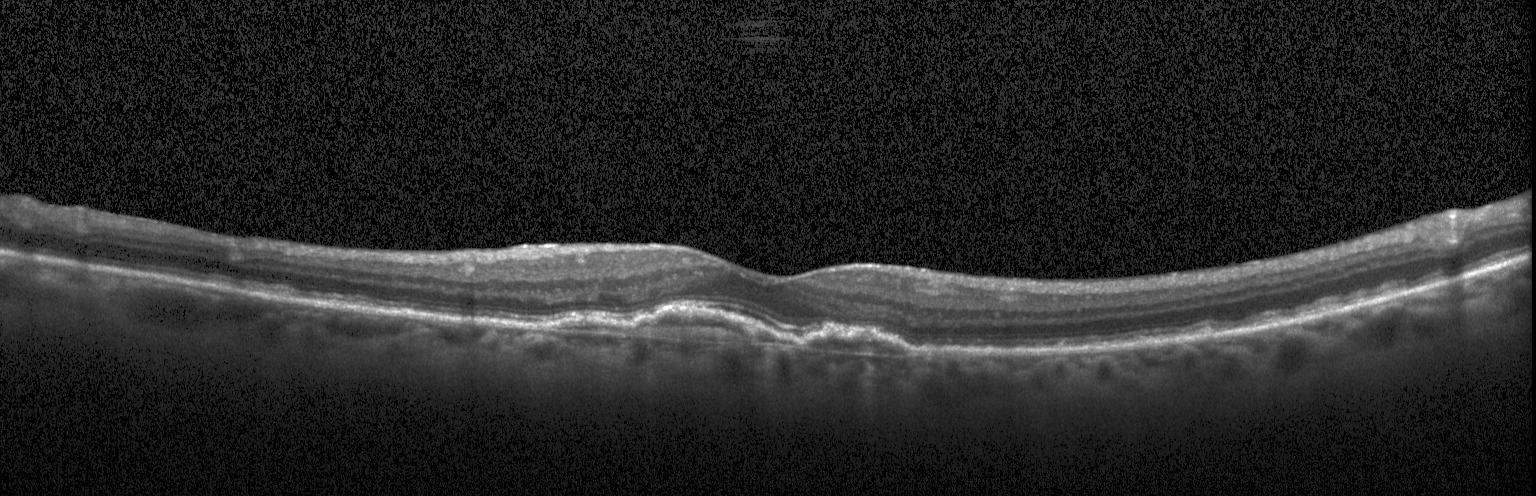

Optical coherence tomography B-scan, horizontal scan through the fovea, SD-OCT.
This B-scan demonstrates a choroidal neovascular membrane.